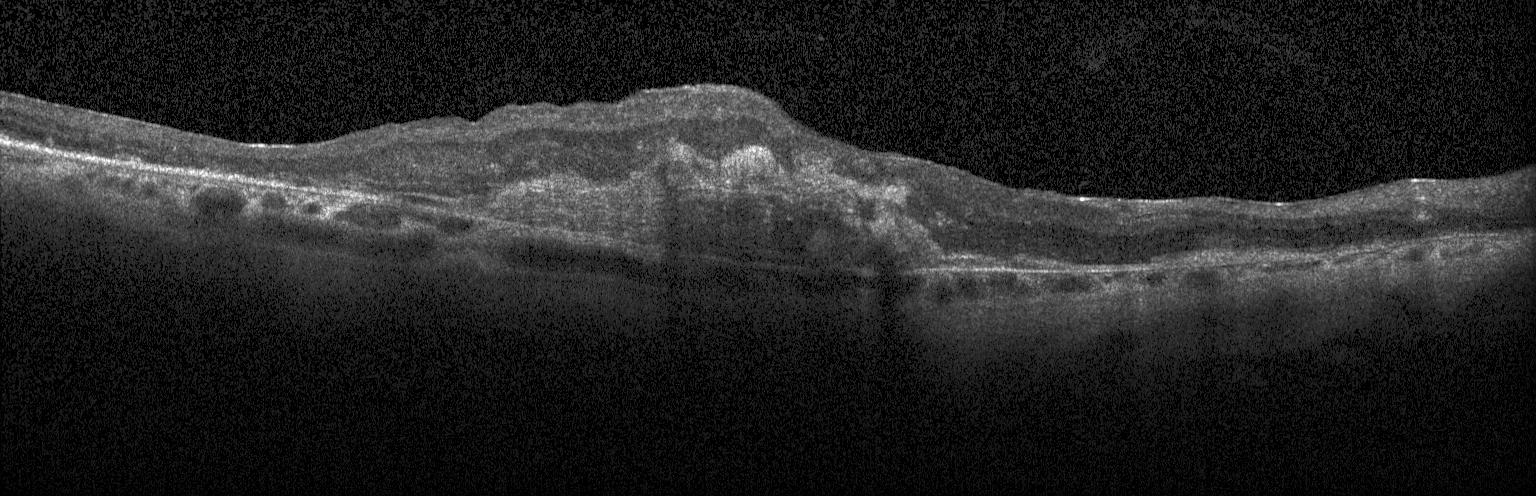

Macular OCT: a choroidal neovascular membrane.